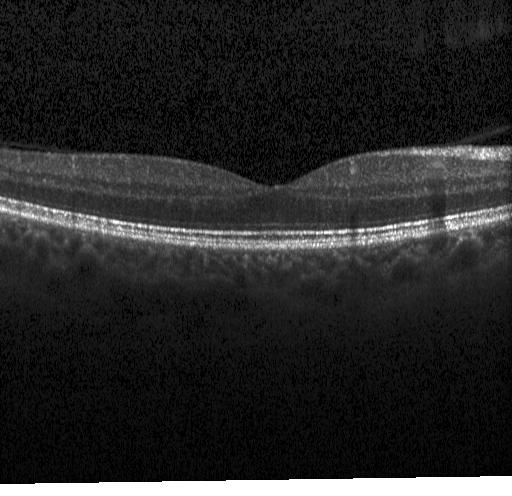

Through the macula · Heidelberg Spectralis · retinal OCT B-scan · spectral-domain OCT — This B-scan demonstrates no choroidal neovascularization, no diabetic macular edema, and no drusen.